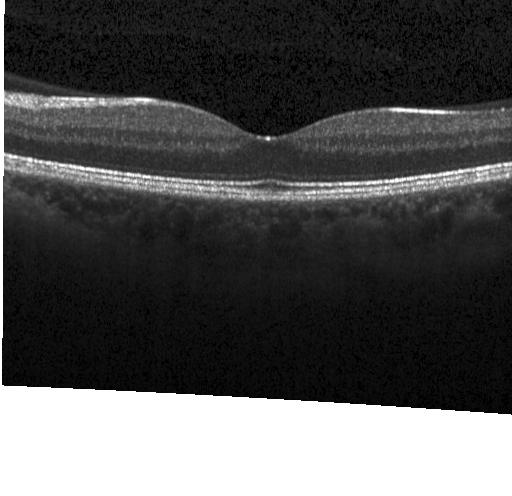

This B-scan demonstrates neither choroidal neovascularization, diabetic macular edema, nor drusen.